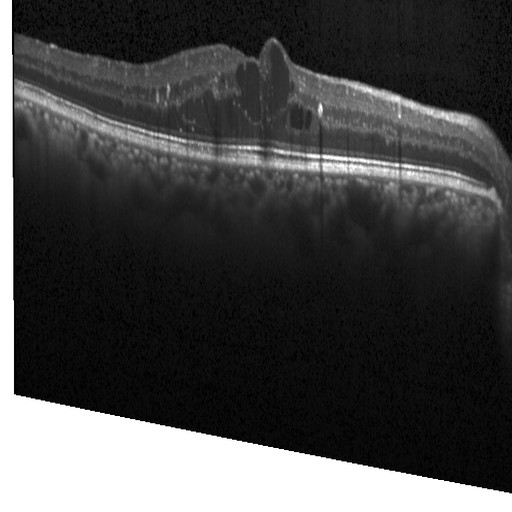 Optical coherence tomography scan. Through the macula. Heidelberg Spectralis. Spectral-domain optical coherence tomography — Macular OCT: DME.